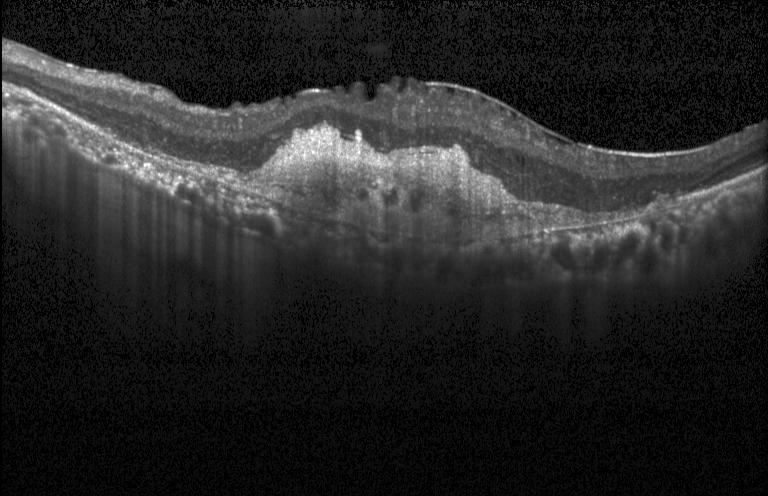 SD-OCT, optical coherence tomography B-scan.
Diagnosis: choroidal neovascularization.